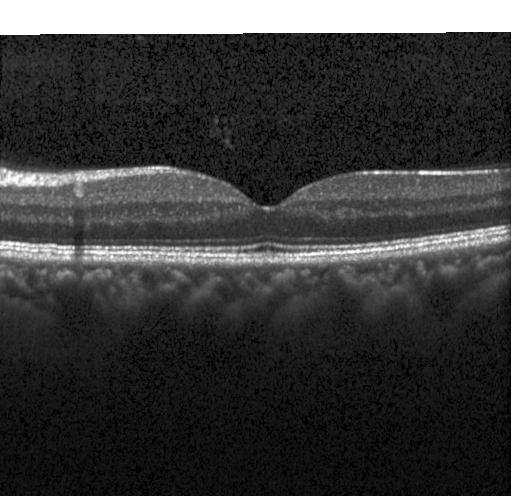
Optical coherence tomography scan — Finding: neither CNV, DME, nor drusen.